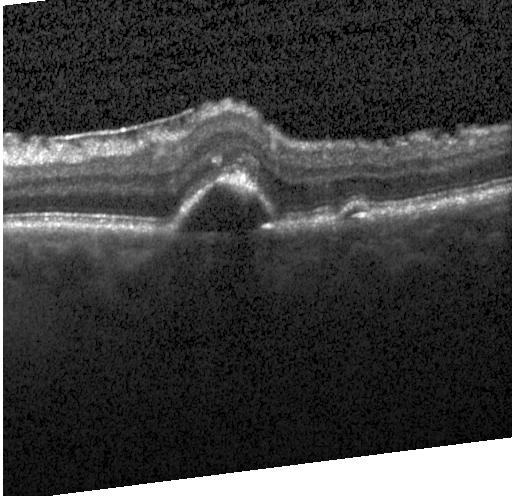
Retinal OCT cross-section showing a choroidal neovascular membrane.